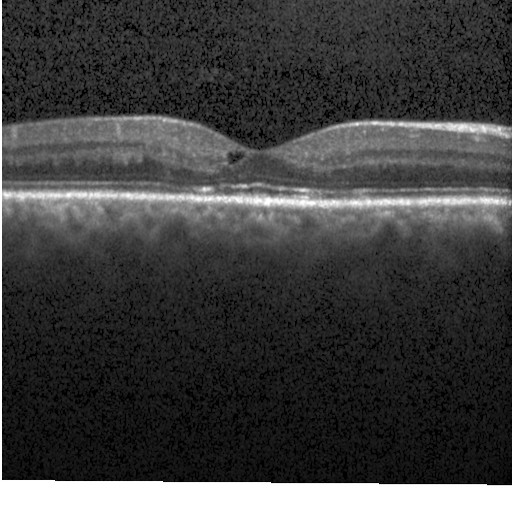
The scan shows diabetic macular edema.